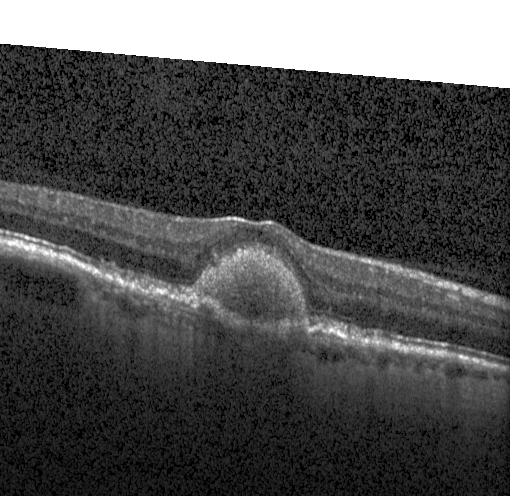 Diagnosis: choroidal neovascularization (CNV).